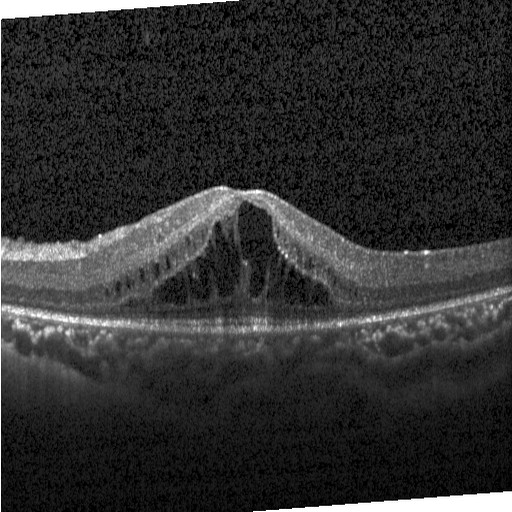 OCT line scan. The scan shows diabetic macular edema (DME).